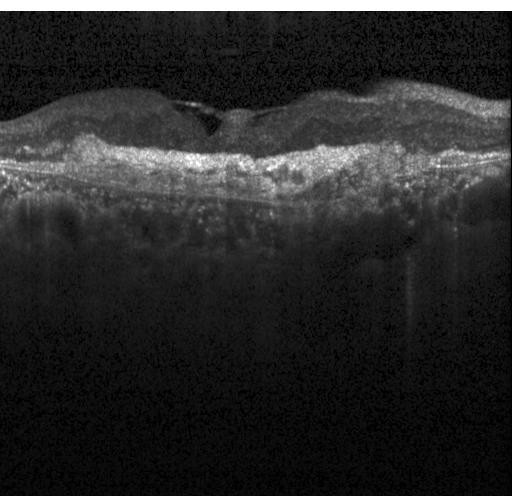 This B-scan demonstrates a choroidal neovascular membrane.